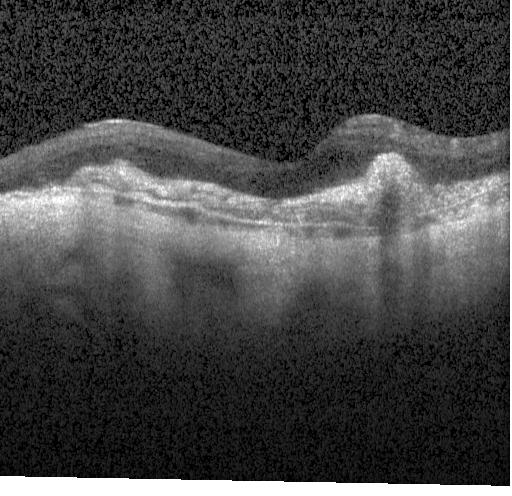

Retinal OCT cross-section showing choroidal neovascularization (CNV).